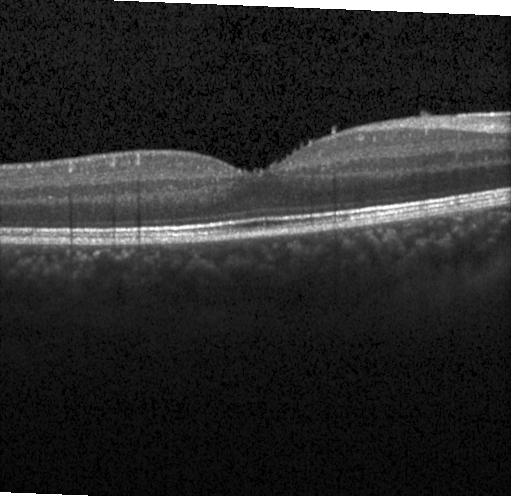 Centered on the fovea, spectral-domain optical coherence tomography, Heidelberg Spectralis OCT system, OCT line scan
Finding: no choroidal neovascularization, no diabetic macular edema, and no drusen.